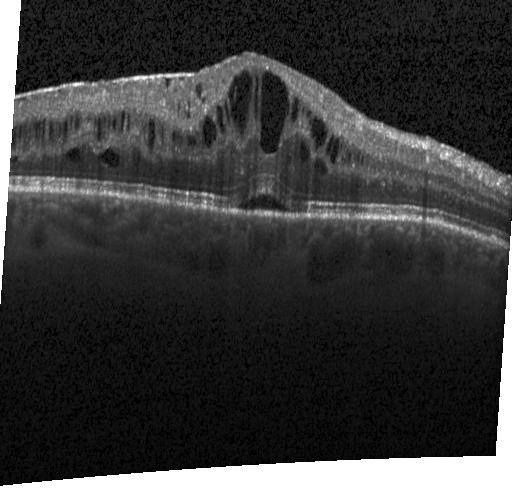 Finding: diabetic macular edema (DME).